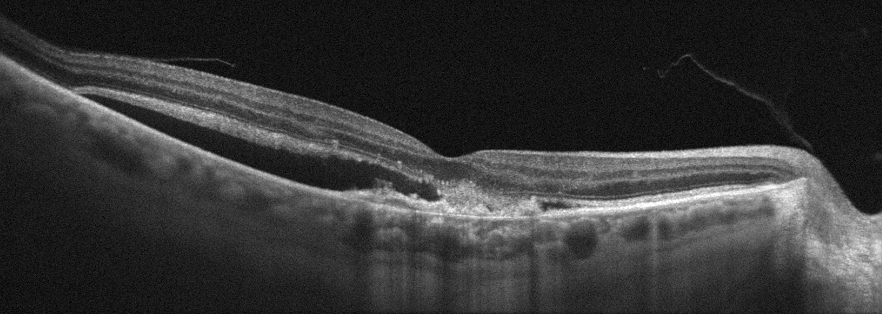 Acquired on an Optovue Avanti RTVue XR, OD, OCT line scan. Diagnosis: age-related macular degeneration (AMD).